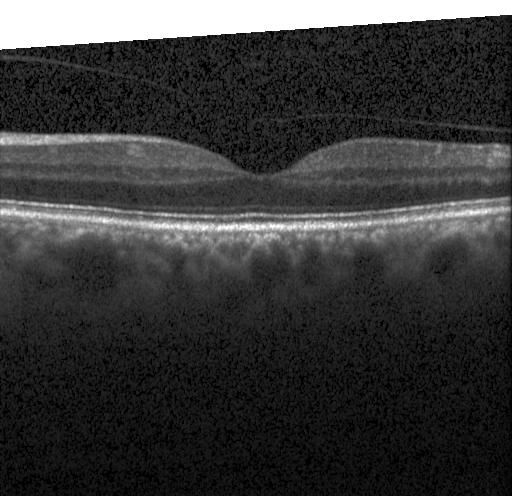
Retinal OCT cross-section showing neither choroidal neovascularization, diabetic macular edema, nor drusen.